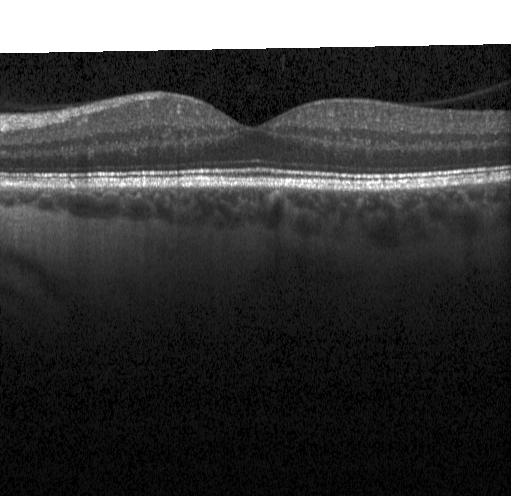

Retinal OCT cross-section · instrument: Heidelberg Spectralis · through the macula · SD-OCT.
Diagnosis: neither choroidal neovascularization, diabetic macular edema, nor drusen.